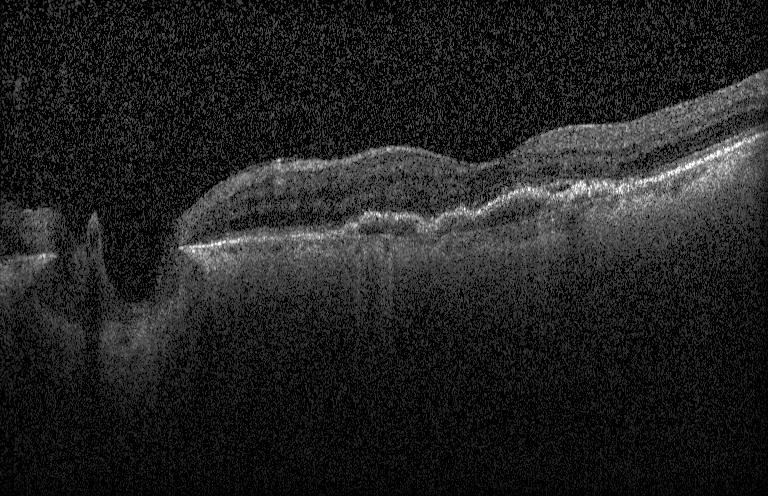 SD-OCT, retinal OCT B-scan.
Diagnosis: a choroidal neovascular membrane.